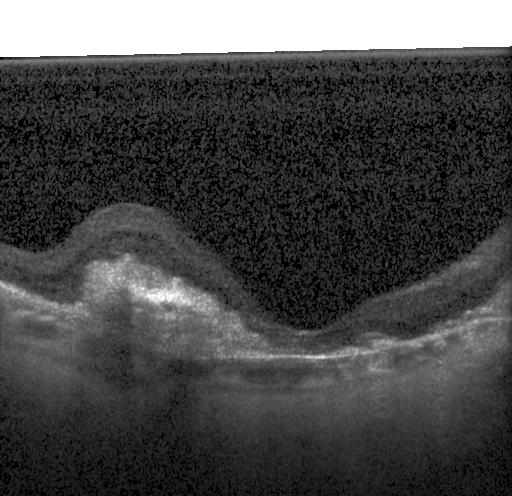 Finding: a choroidal neovascular membrane.